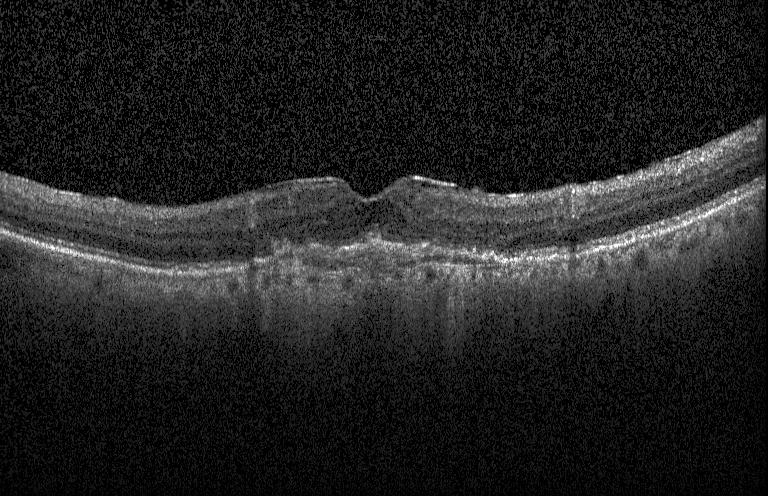 Heidelberg Spectralis; retinal OCT B-scan; spectral-domain OCT. Finding: a choroidal neovascular membrane.